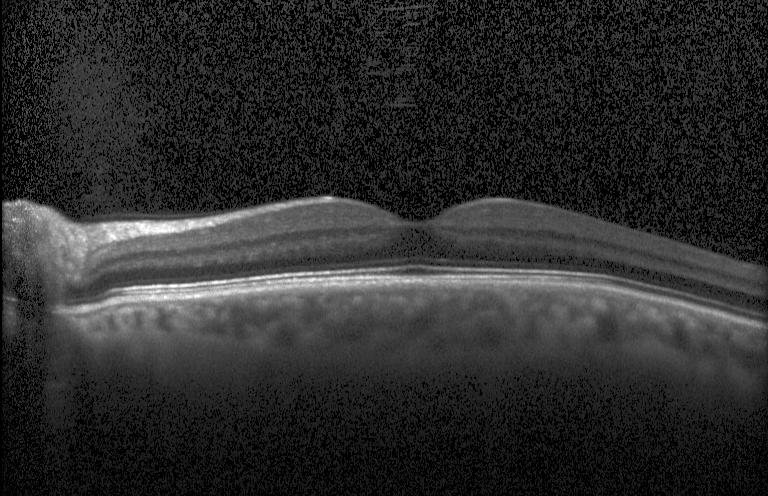 OCT B-scan.
The scan shows no choroidal neovascularization, no diabetic macular edema, and no drusen.